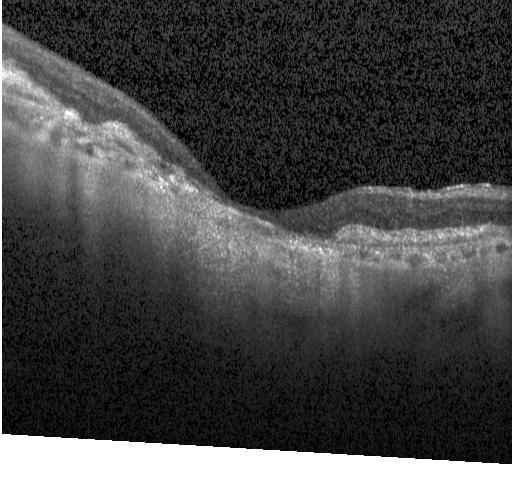 Macular OCT demonstrating a choroidal neovascular membrane.